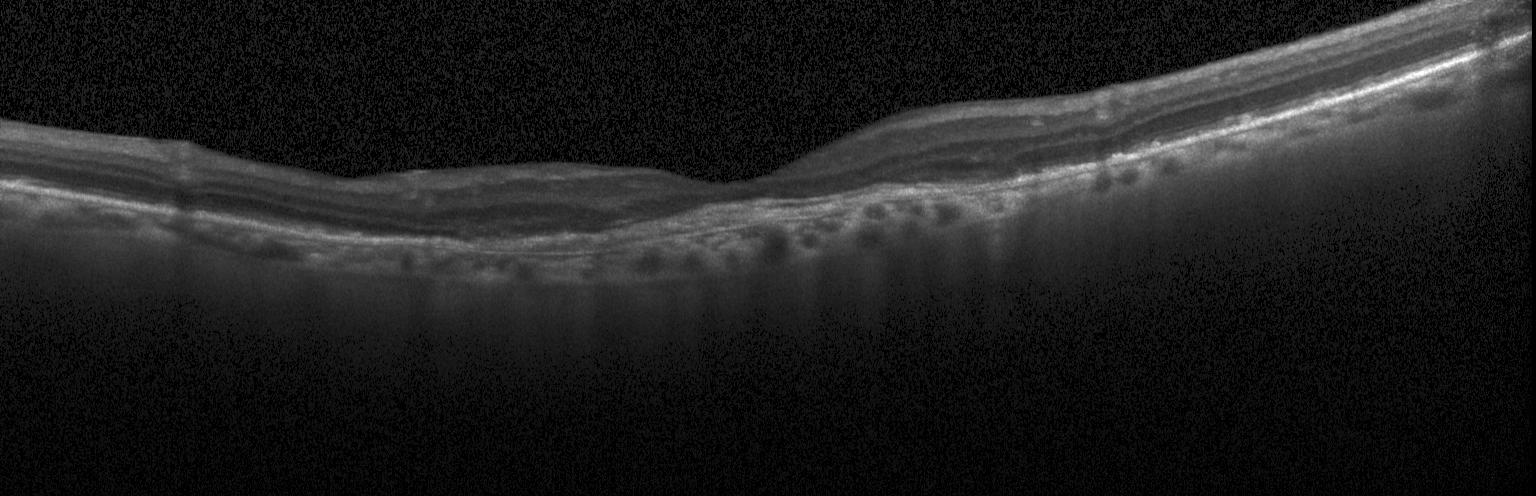 The scan shows a choroidal neovascular membrane.